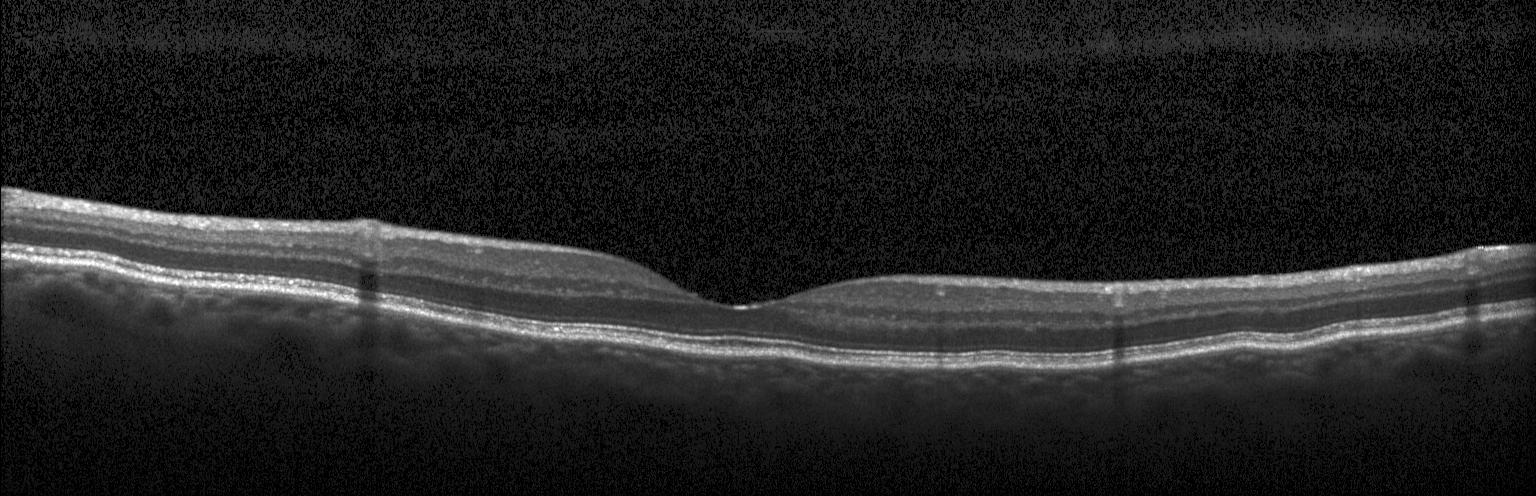

Retinal OCT B-scan
Finding: no evidence of choroidal neovascularization, diabetic macular edema, or drusen.